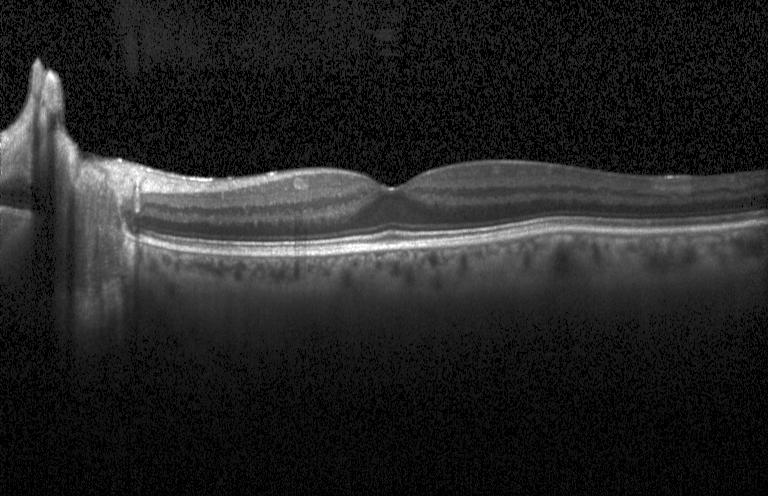 No choroidal neovascularization, diabetic macular edema, or drusen.